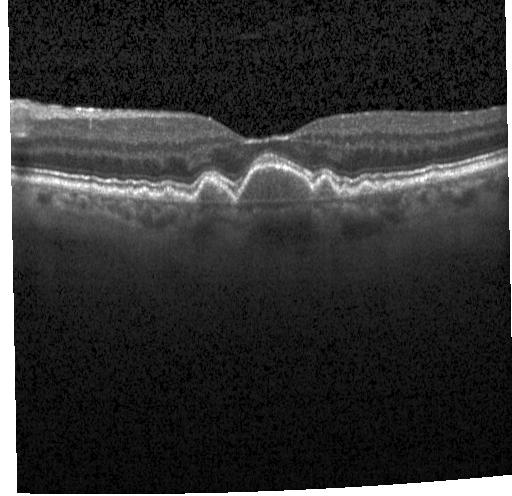 Spectral-domain OCT · Heidelberg Spectralis OCT system · optical coherence tomography B-scan — This B-scan demonstrates drusen.